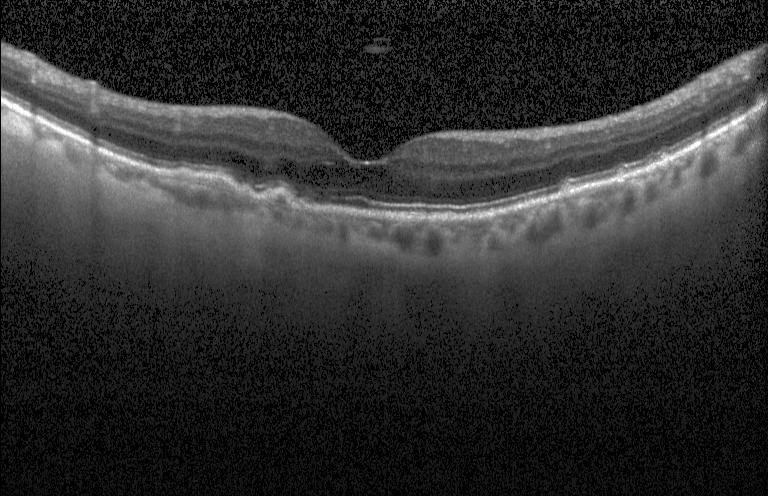
Impression: choroidal neovascularization (CNV).